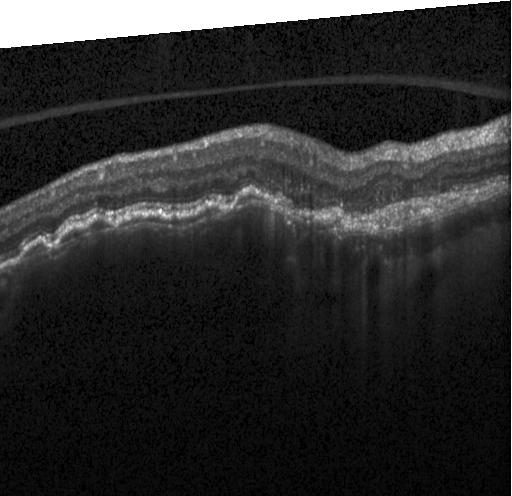

Retinal OCT cross-section. Macular OCT: choroidal neovascularization (CNV).